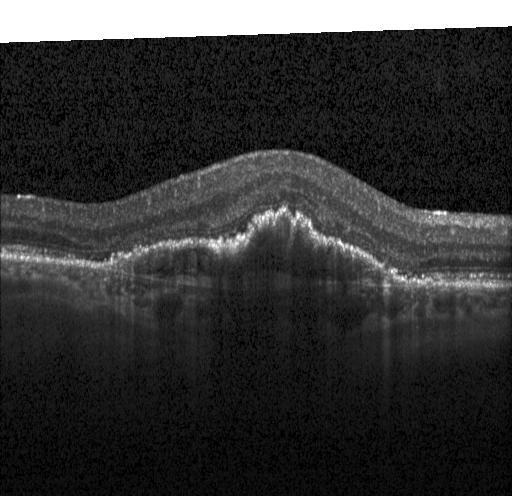 Acquired on a Heidelberg Spectralis, optical coherence tomography B-scan, SD-OCT.
The scan shows choroidal neovascularization (CNV).